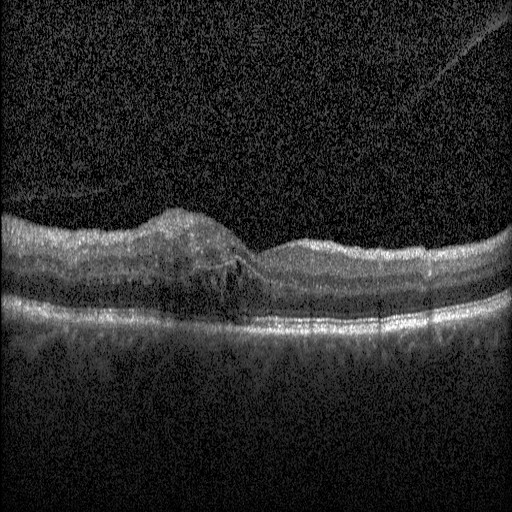

Fovea-centered, spectral-domain optical coherence tomography, Heidelberg Spectralis OCT system, retinal OCT cross-section.
Finding: diabetic macular edema (DME).